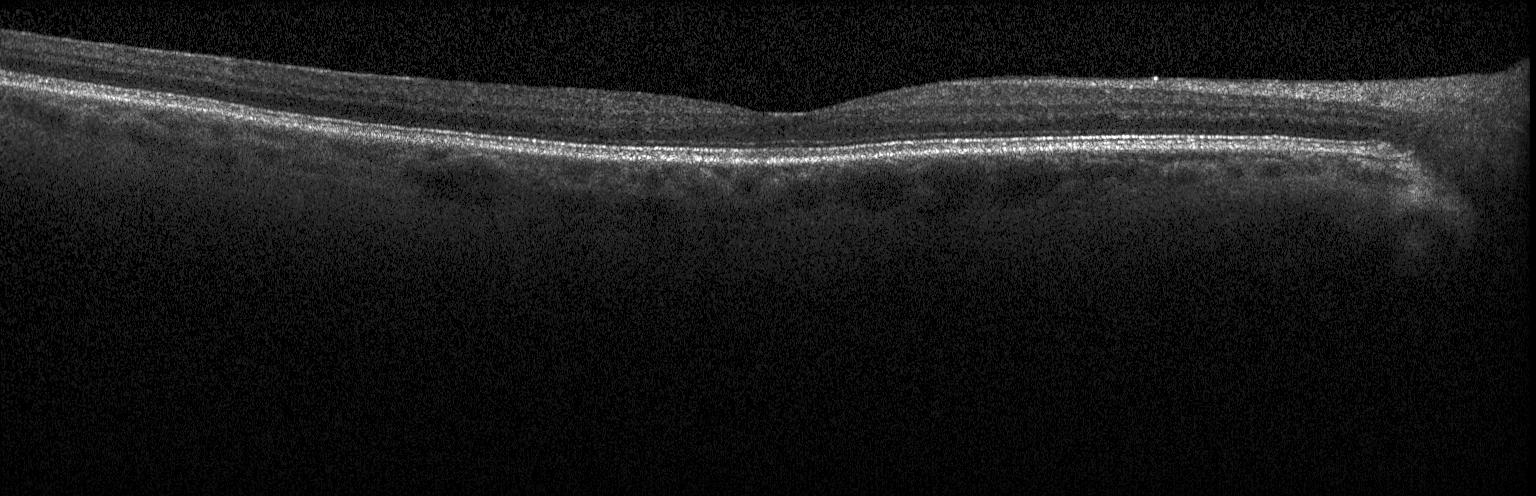

Retinal OCT B-scan · Heidelberg Spectralis OCT system — OCT finding: no CNV, DME, or drusen.